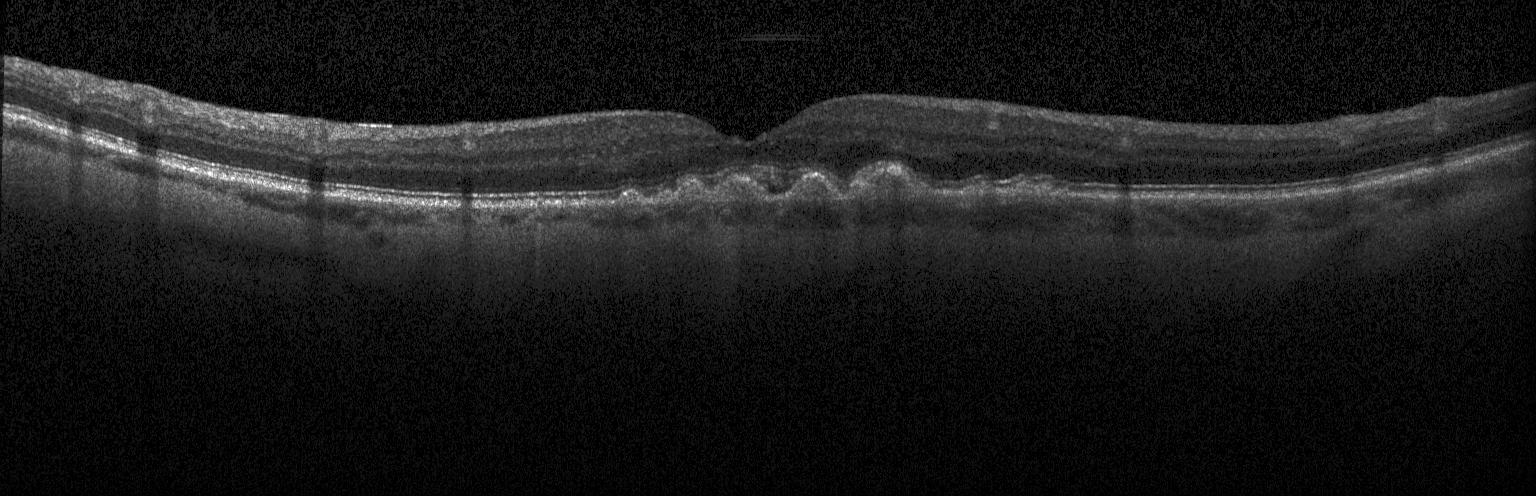 Retinal OCT cross-section.
Impression: drusen.